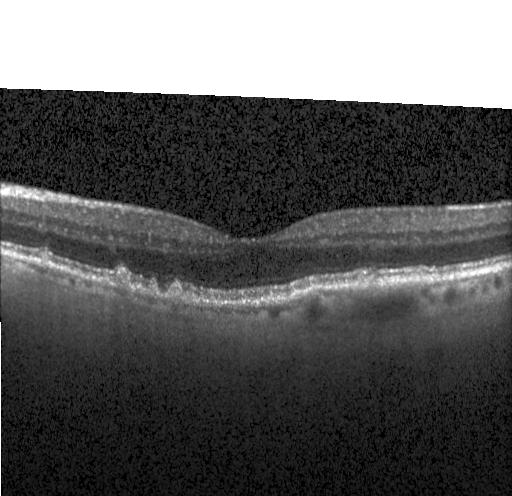
Retinal OCT B-scan
This B-scan demonstrates sub-RPE drusenoid deposits.